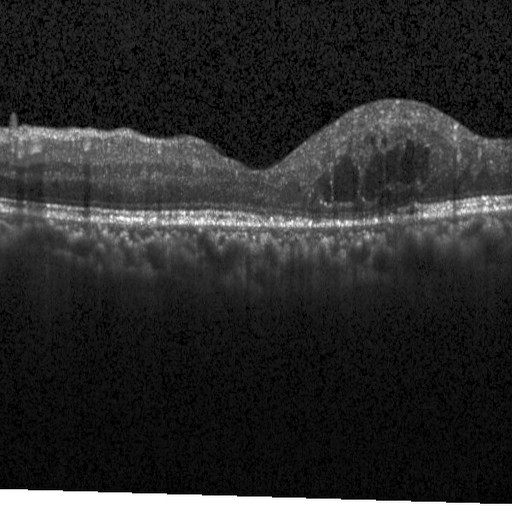

OCT B-scan showing diabetic macular edema (DME).